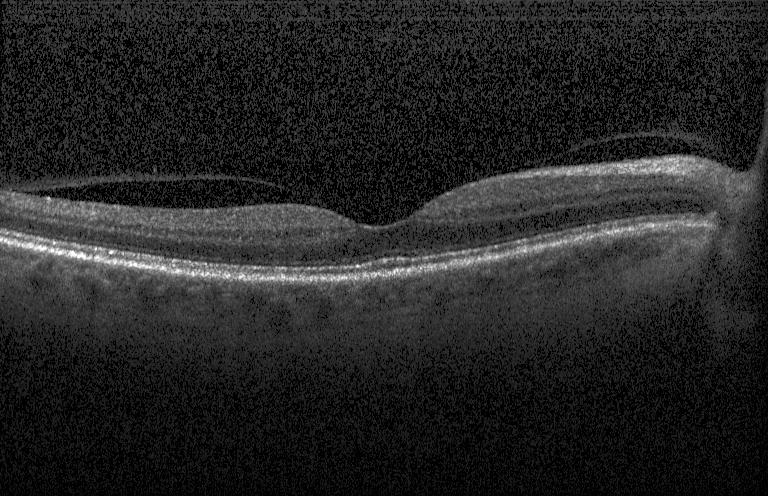

The scan shows no choroidal neovascularization, diabetic macular edema, or drusen.